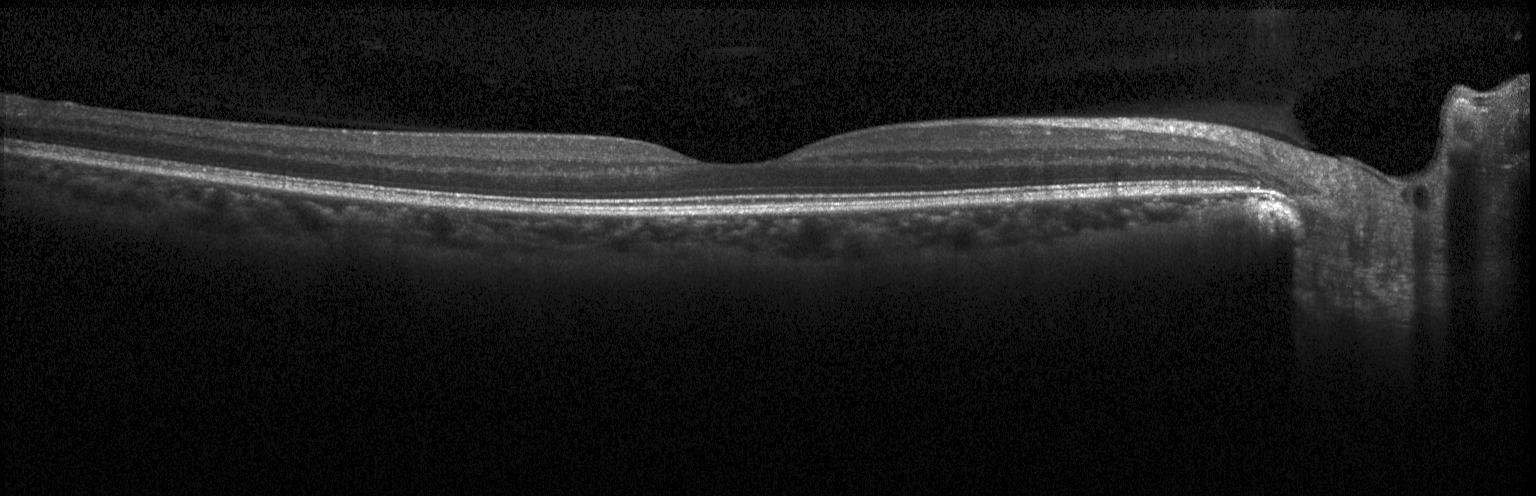

Spectral-domain OCT; OCT line scan.
Assessment: neither choroidal neovascularization, diabetic macular edema, nor drusen.